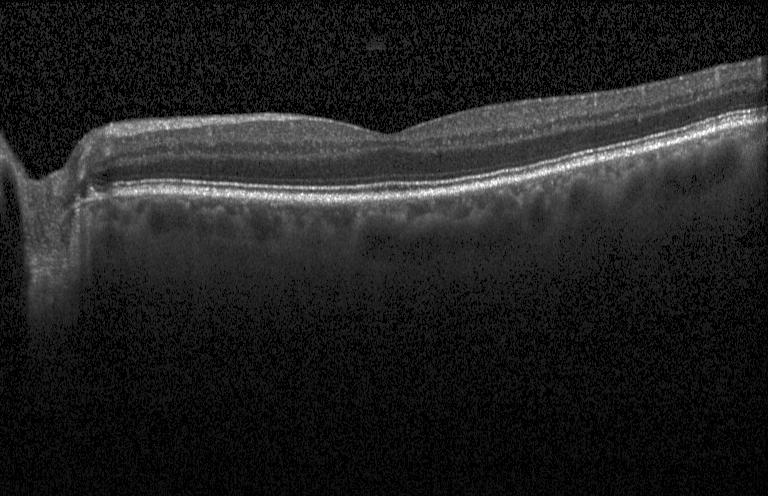

Heidelberg Spectralis OCT system; optical coherence tomography scan; macular scan; spectral-domain optical coherence tomography — Diagnosis: no evidence of choroidal neovascularization, diabetic macular edema, or drusen.